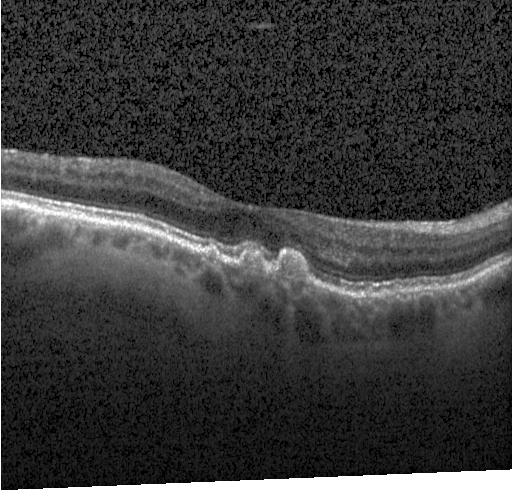
Acquired on a Heidelberg Spectralis · fovea-centered · retinal OCT cross-section — Macular OCT: multiple drusen.